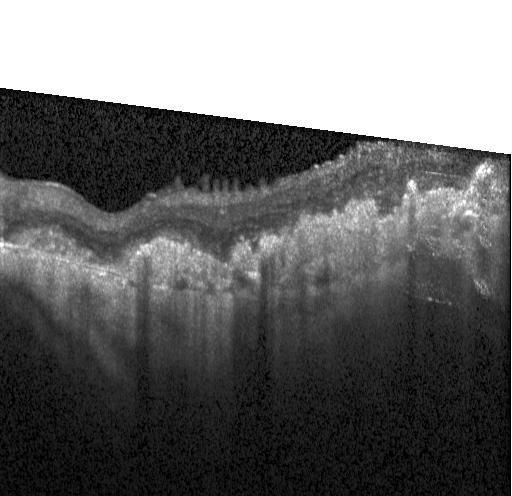 Retinal OCT cross-section
A choroidal neovascular membrane.